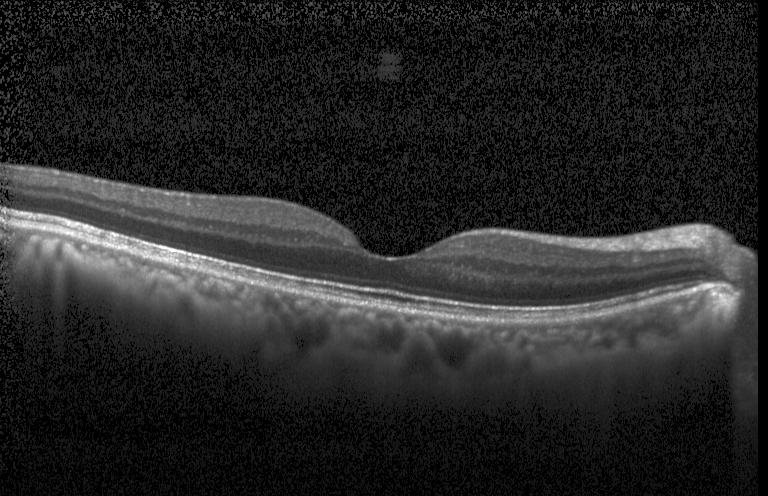 Heidelberg Spectralis. SD-OCT. Centered on the fovea. Optical coherence tomography B-scan. Diagnosis: no CNV, DME, or drusen.